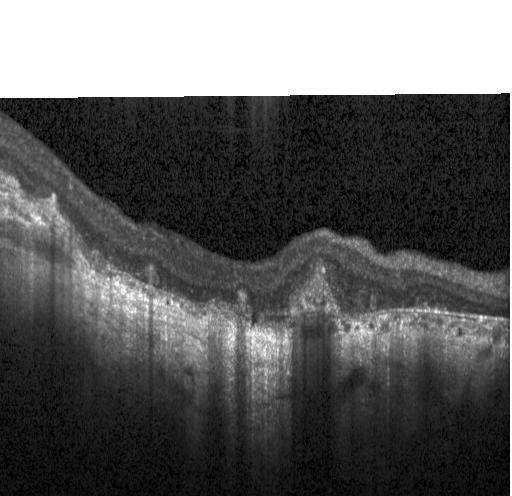 SD-OCT, fovea-centered, optical coherence tomography B-scan.
Finding: a choroidal neovascular membrane.